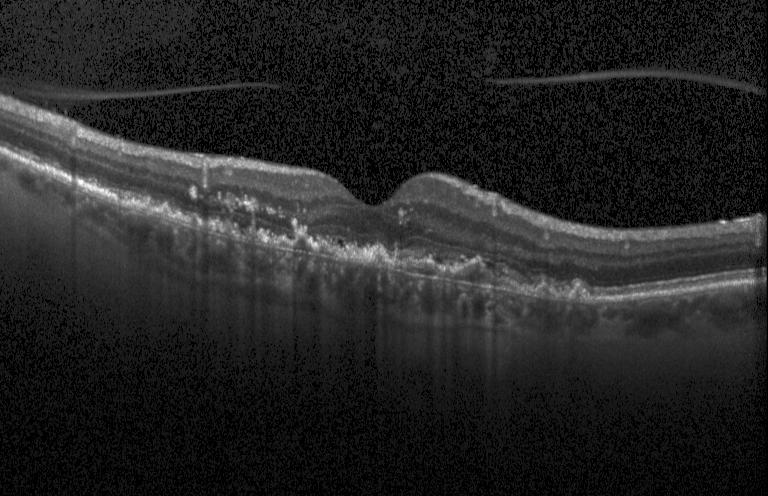 OCT scan showing a choroidal neovascular membrane.